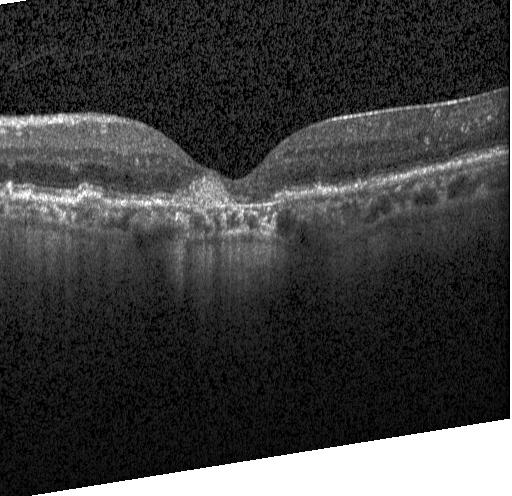 Dx: choroidal neovascularization (CNV).